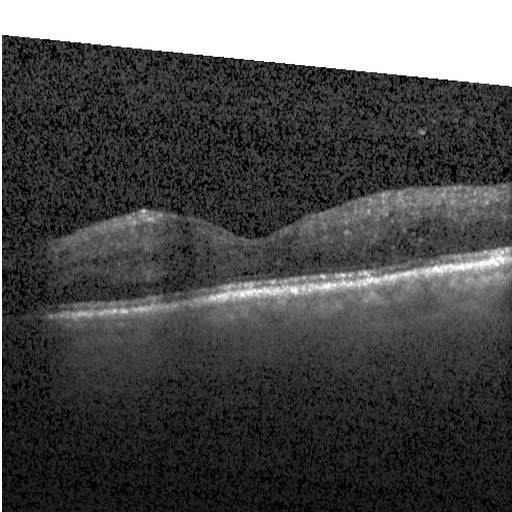 Retinal OCT cross-section. Diabetic macular edema (DME).